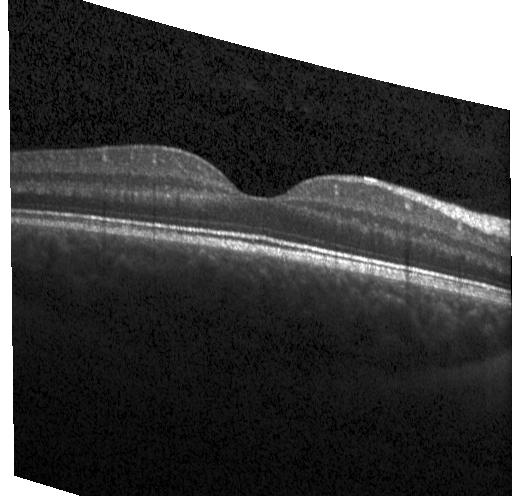 OCT finding: no evidence of CNV, DME, or drusen.